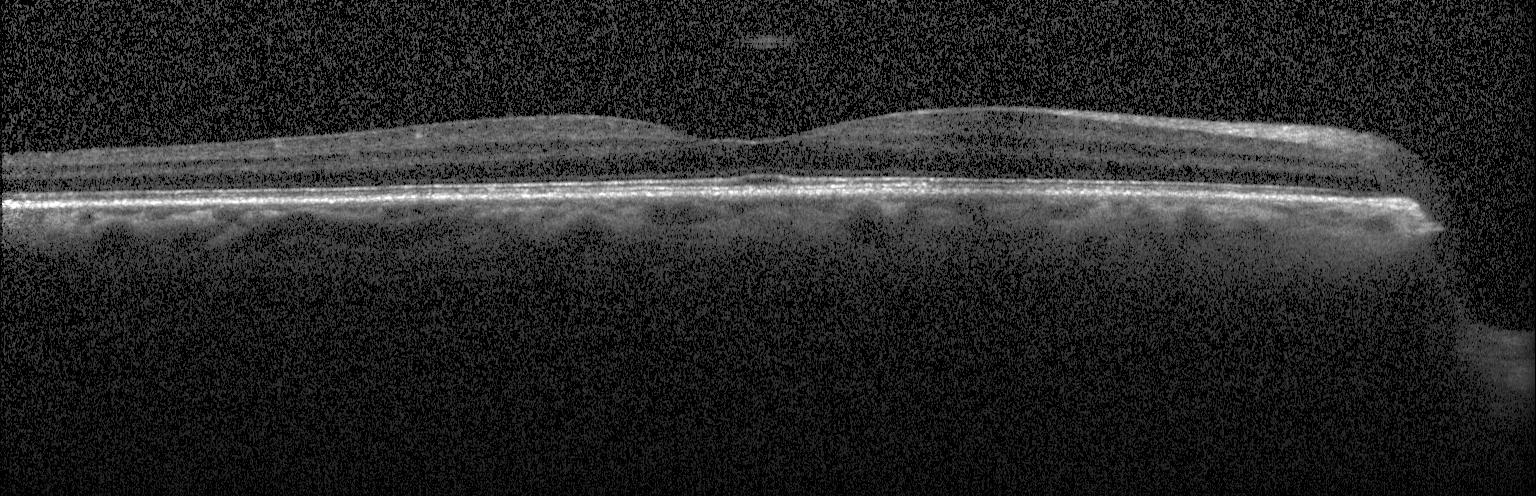
Spectral-domain optical coherence tomography · acquired on a Heidelberg Spectralis · retinal OCT cross-section. Impression: neither choroidal neovascularization, diabetic macular edema, nor drusen.